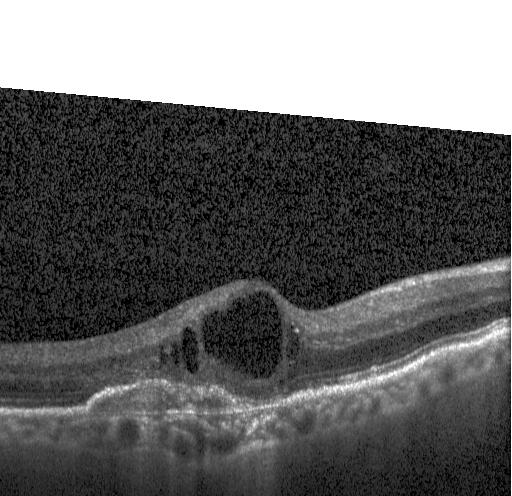
Heidelberg Spectralis OCT system, horizontal scan through the fovea, retinal OCT B-scan, spectral-domain optical coherence tomography — Impression: a choroidal neovascular membrane.